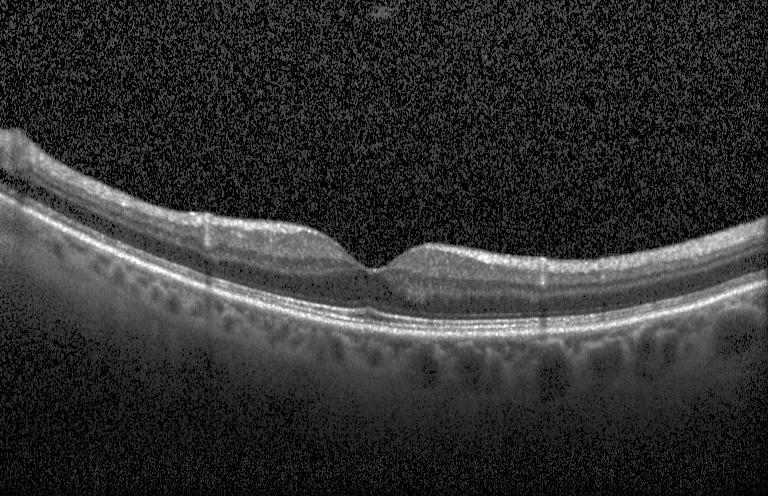
SD-OCT; macular scan; retinal OCT B-scan; acquired on a Heidelberg Spectralis. Diagnosis: no choroidal neovascularization, diabetic macular edema, or drusen.